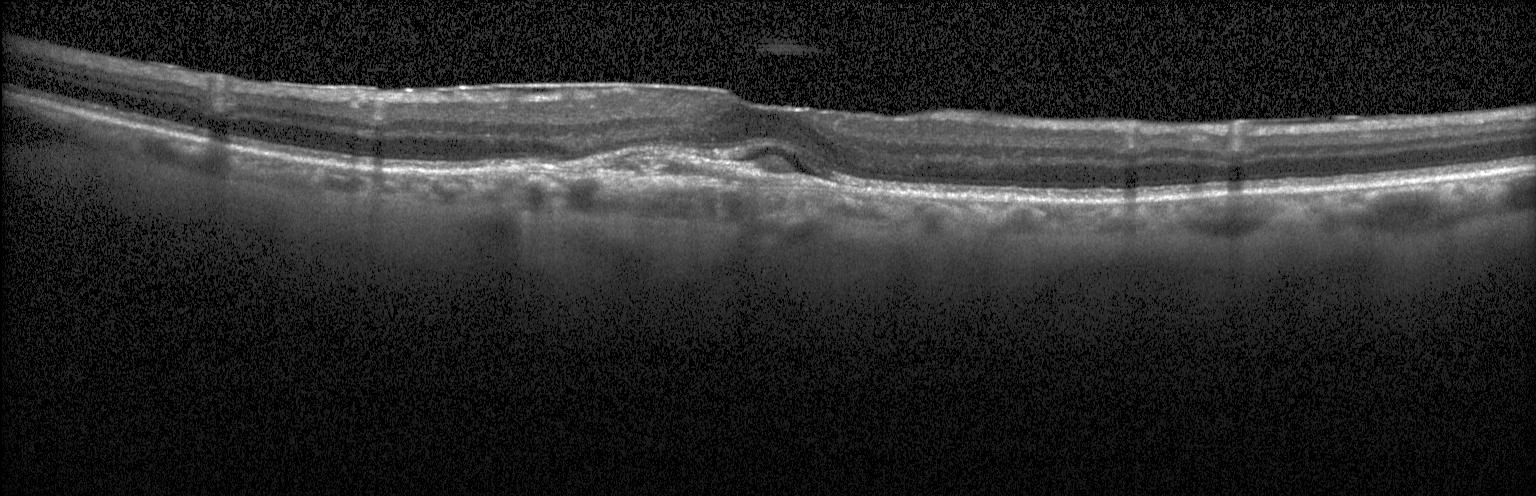
Spectral-domain optical coherence tomography. Through the macula. Optical coherence tomography B-scan. OCT finding: a choroidal neovascular membrane.